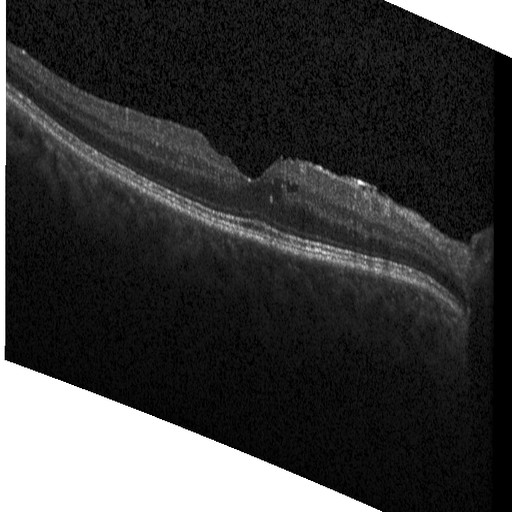
Macular OCT: diabetic macular edema (DME).